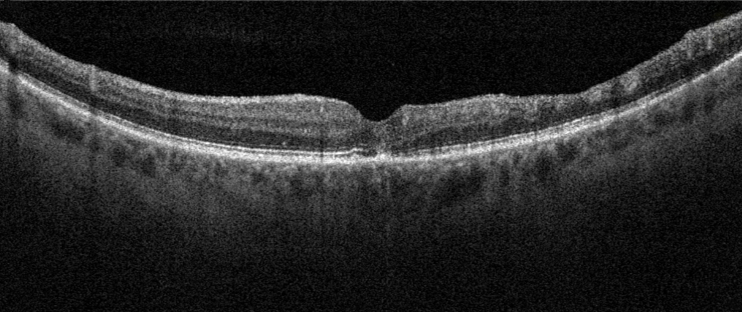

Assessment: diabetic macular edema (DME).